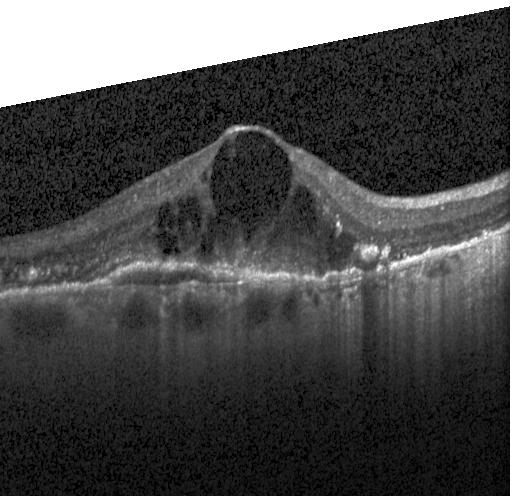

Horizontal scan through the fovea · OCT line scan · spectral-domain optical coherence tomography.
Impression: a choroidal neovascular membrane.